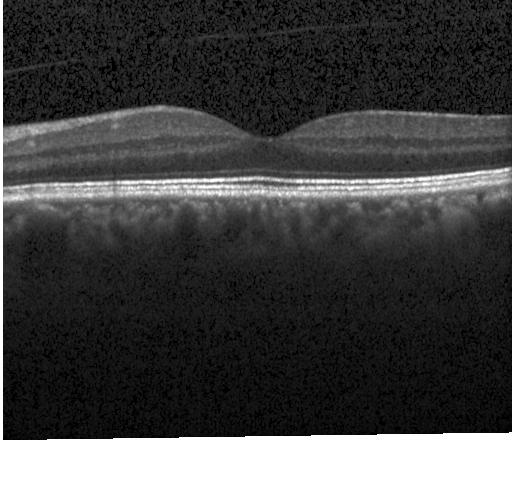

Macular OCT: no choroidal neovascularization, diabetic macular edema, or drusen.